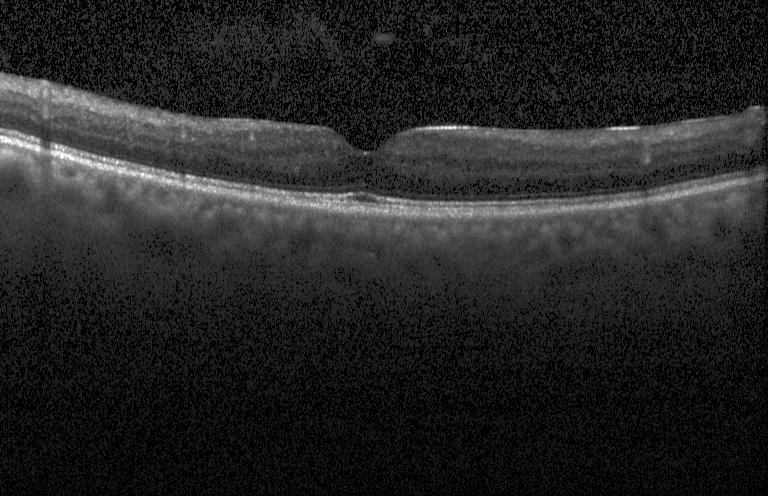
Retinal OCT B-scan; SD-OCT. Impression: no choroidal neovascularization, diabetic macular edema, or drusen.